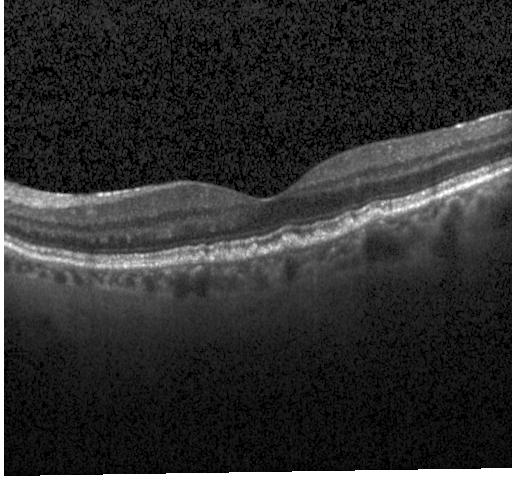 Finding: multiple drusen.